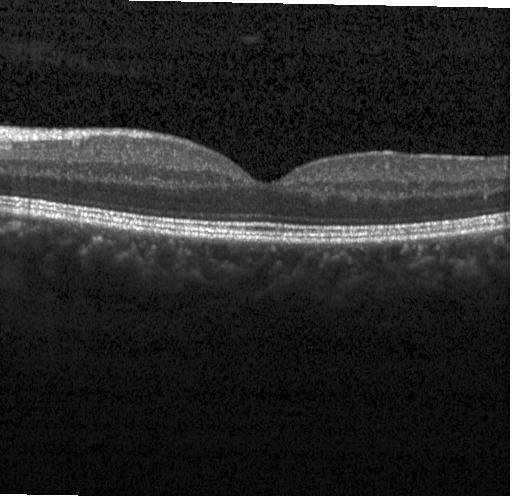

Retinal OCT cross-section, acquired on a Heidelberg Spectralis, through the macula, spectral-domain optical coherence tomography.
Assessment: no evidence of CNV, DME, or drusen.